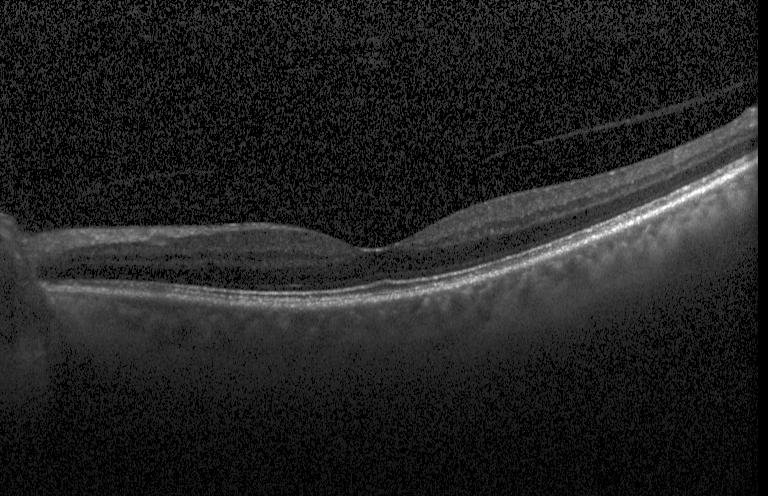

Through the macula. Spectral-domain optical coherence tomography. Optical coherence tomography scan. Heidelberg Spectralis OCT system — This B-scan demonstrates no evidence of choroidal neovascularization, diabetic macular edema, or drusen.